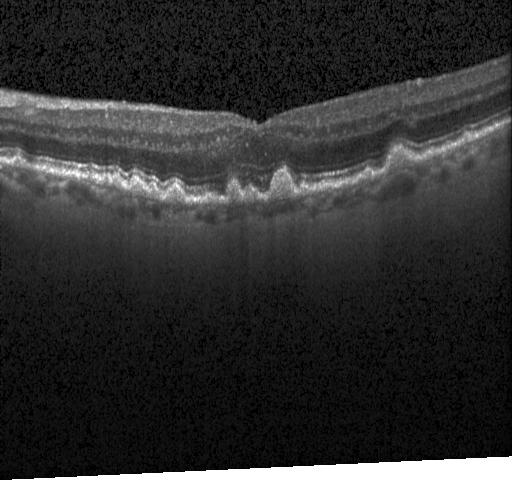
Retinal OCT B-scan · SD-OCT · acquired on a Heidelberg Spectralis · horizontal scan through the fovea.
Macular OCT: sub-RPE drusenoid deposits.